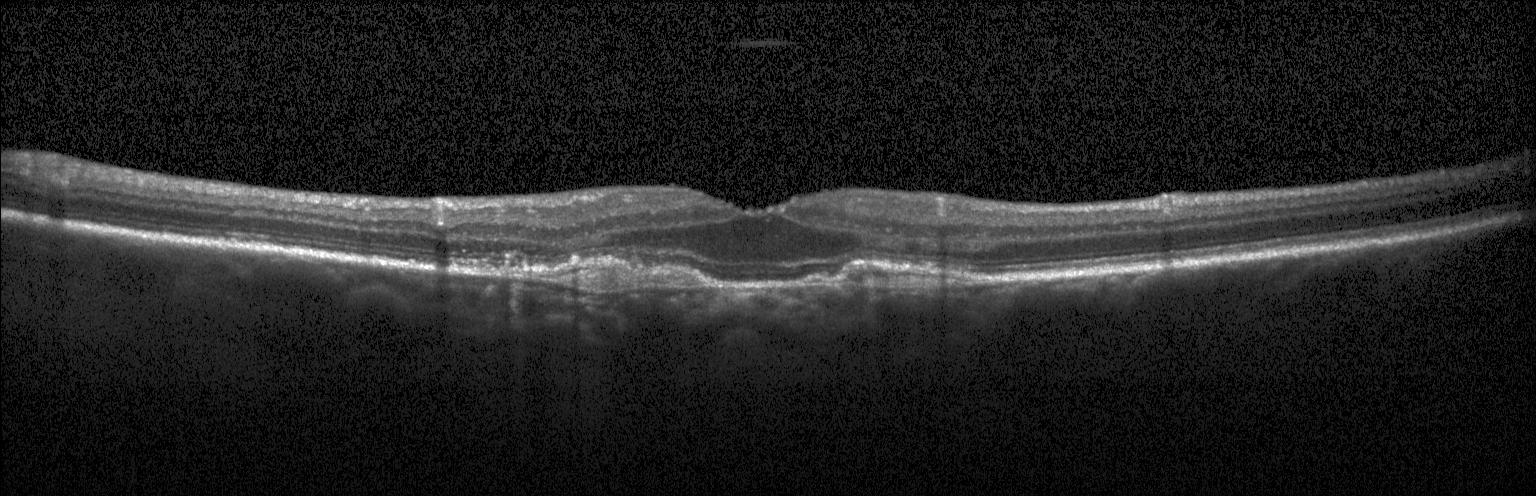
Diagnosis: a choroidal neovascular membrane.